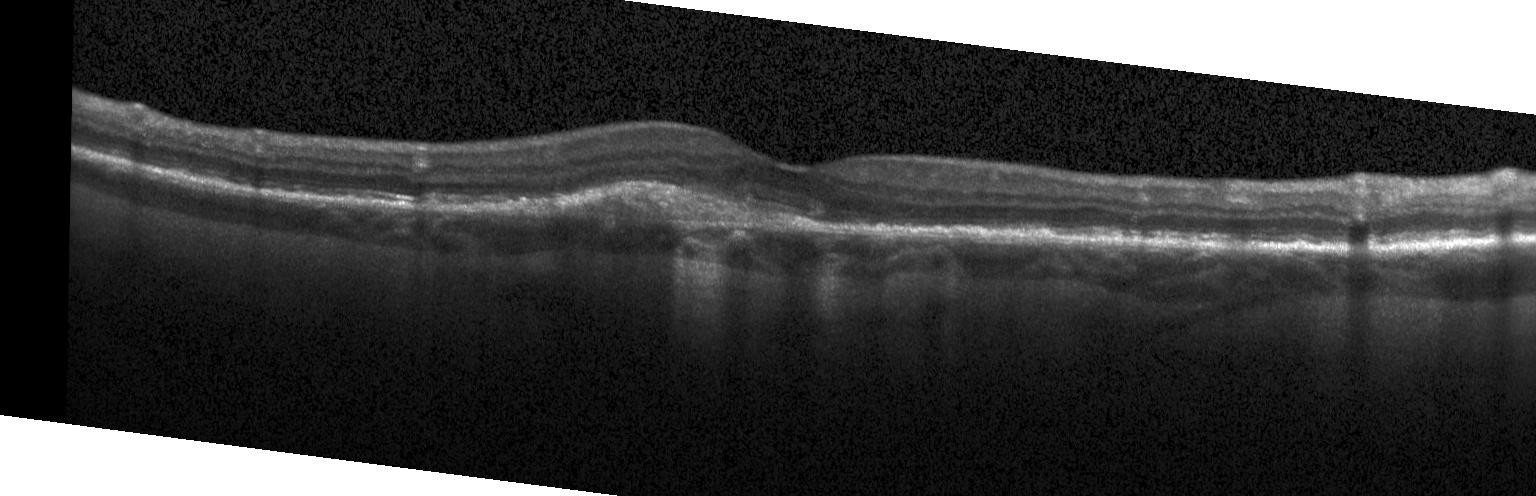 OCT B-scan, Heidelberg Spectralis OCT system, centered on the fovea. Impression: choroidal neovascularization.